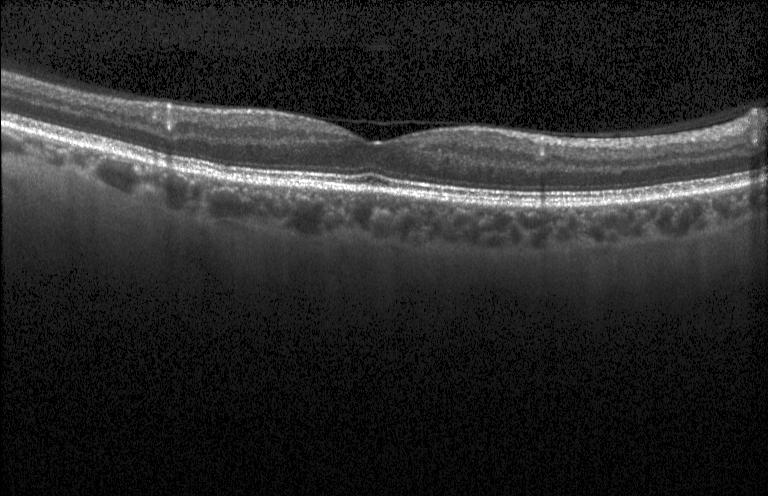

Macular scan; Heidelberg Spectralis OCT system; optical coherence tomography scan. Macular OCT: no choroidal neovascularization, no diabetic macular edema, and no drusen.